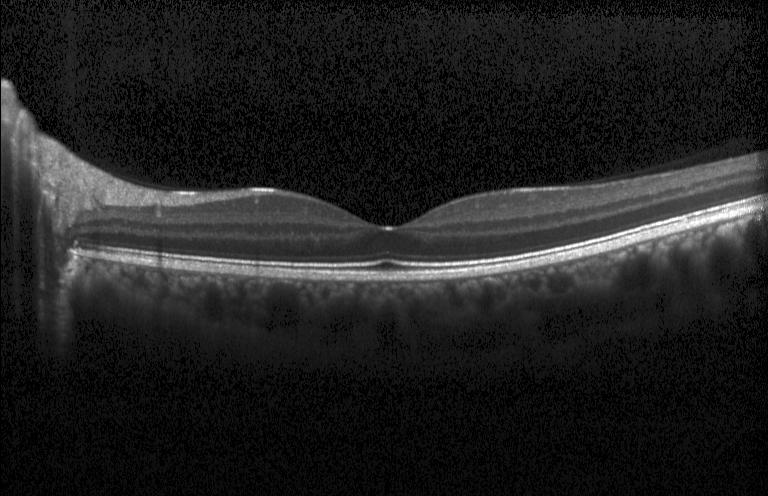 OCT B-scan showing no choroidal neovascularization, no diabetic macular edema, and no drusen.